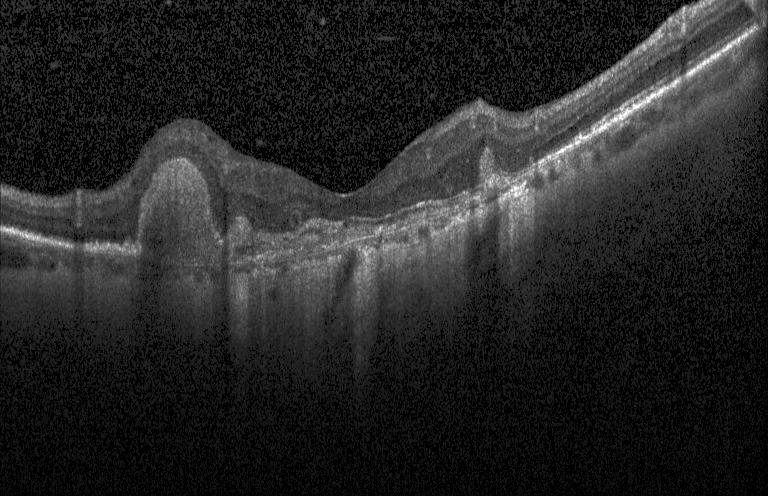 Optical coherence tomography B-scan.
A choroidal neovascular membrane.